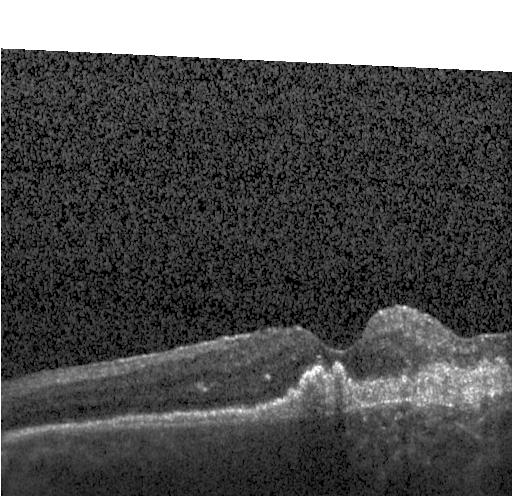

Retinal OCT cross-section; Heidelberg Spectralis
Impression: choroidal neovascularization.